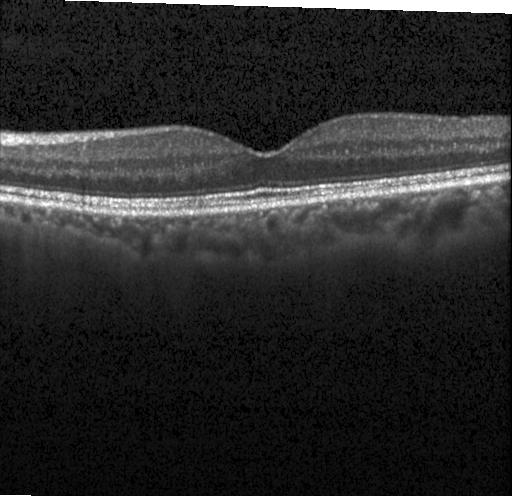
Optical coherence tomography B-scan — Diagnosis: neither choroidal neovascularization, diabetic macular edema, nor drusen.